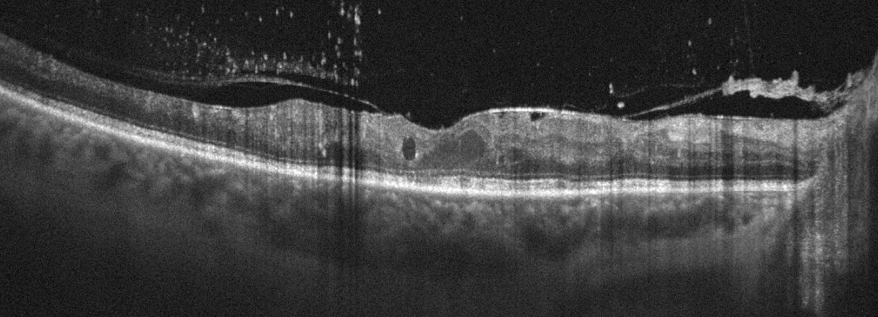

Optical coherence tomography B-scan — OCT finding: diabetic macular edema (DME).